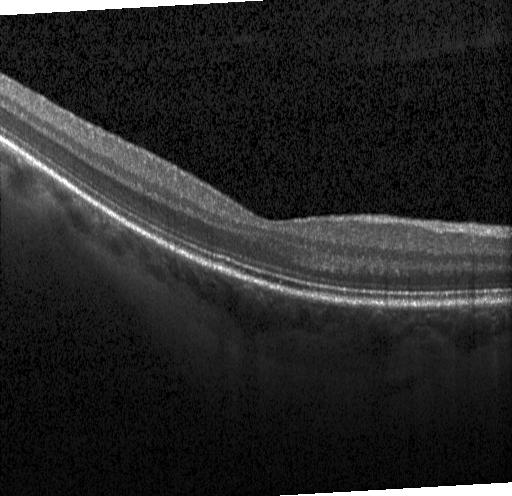
Assessment: no evidence of choroidal neovascularization, diabetic macular edema, or drusen.